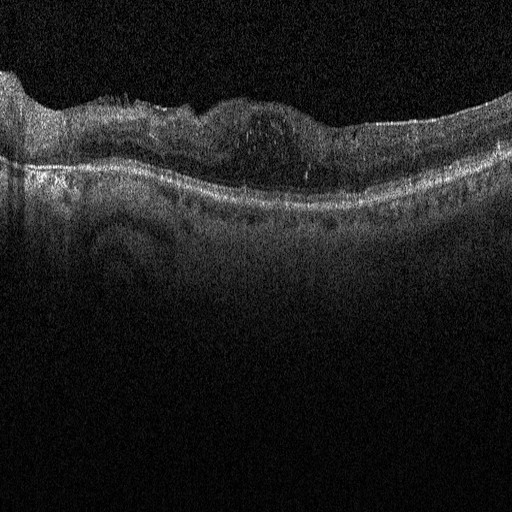

Heidelberg Spectralis · OCT B-scan · spectral-domain optical coherence tomography. This B-scan demonstrates diabetic macular edema.